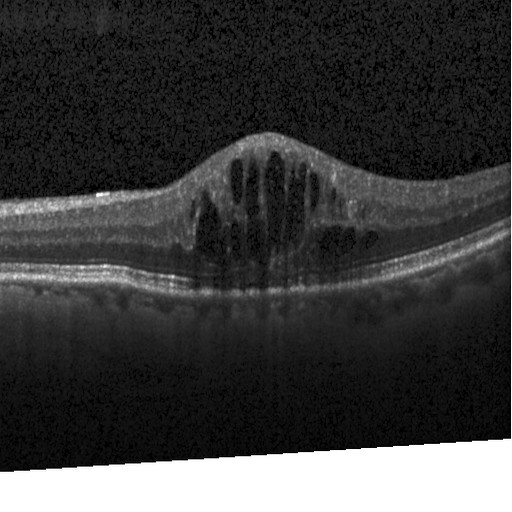

OCT B-scan; macular scan. Macular OCT: DME.